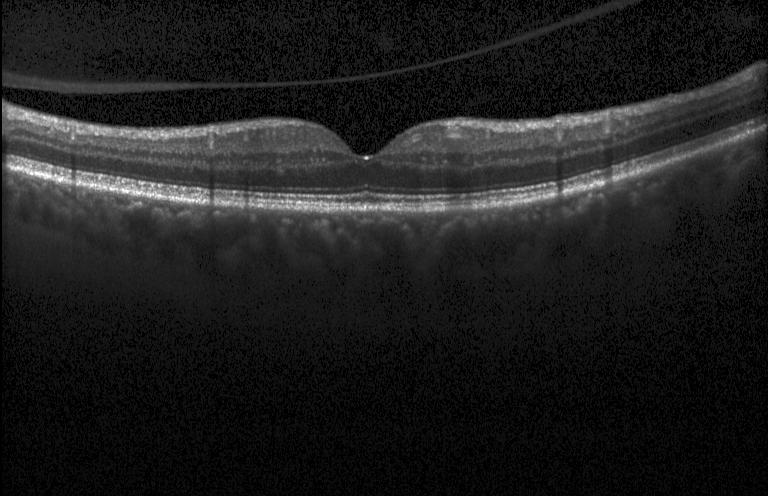

Macular scan, spectral-domain OCT, retinal OCT cross-section, acquired on a Heidelberg Spectralis
No choroidal neovascularization, diabetic macular edema, or drusen.